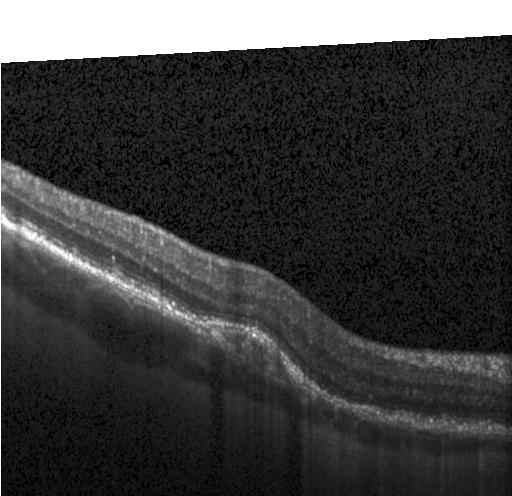 Retinal OCT B-scan, SD-OCT, instrument: Heidelberg Spectralis
The scan shows a choroidal neovascular membrane.